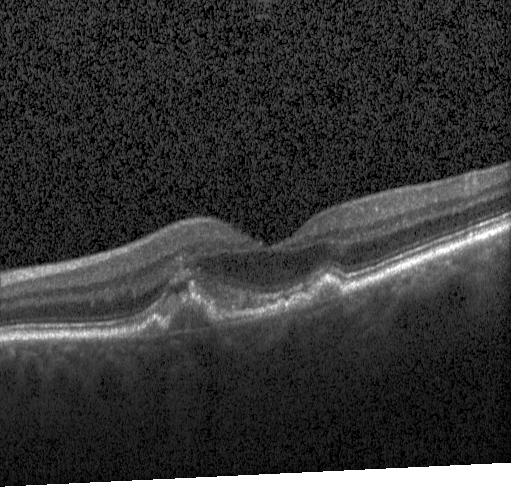
Retinal OCT cross-section.
Impression: choroidal neovascularization (CNV).